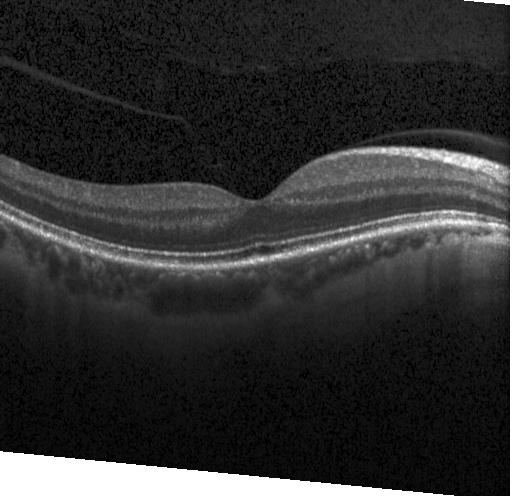
OCT line scan, centered on the fovea
The scan shows neither choroidal neovascularization, diabetic macular edema, nor drusen.